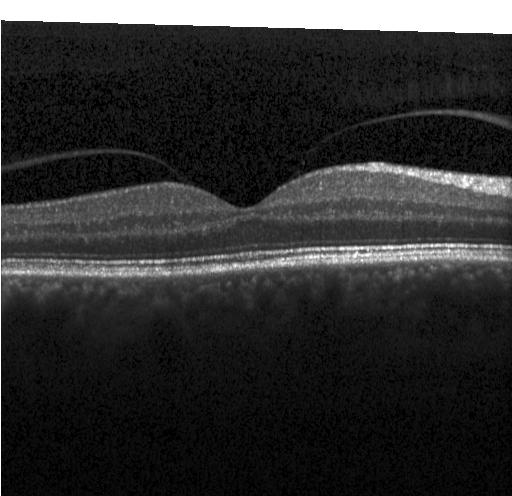 OCT B-scan. Heidelberg Spectralis OCT system. Impression: no evidence of CNV, DME, or drusen.